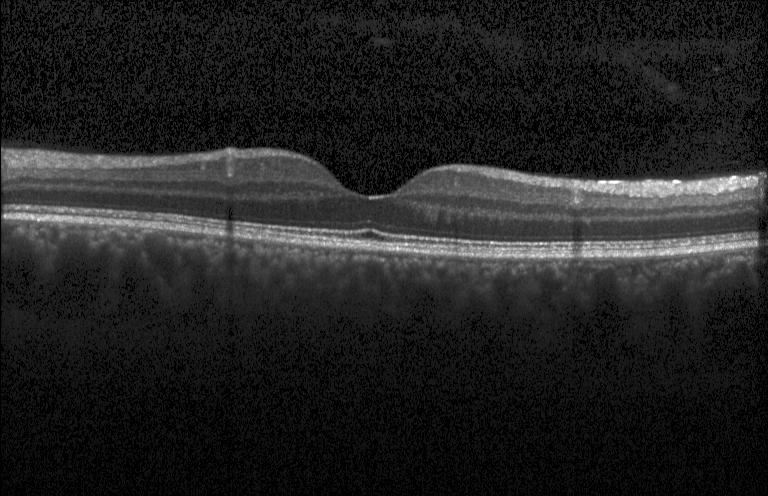

Heidelberg Spectralis OCT system. Centered on the fovea. Retinal OCT B-scan. Spectral-domain optical coherence tomography
This B-scan demonstrates neither choroidal neovascularization, diabetic macular edema, nor drusen.